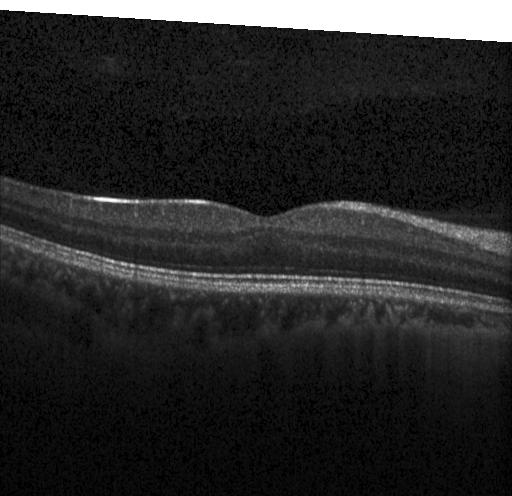
Finding: neither choroidal neovascularization, diabetic macular edema, nor drusen.